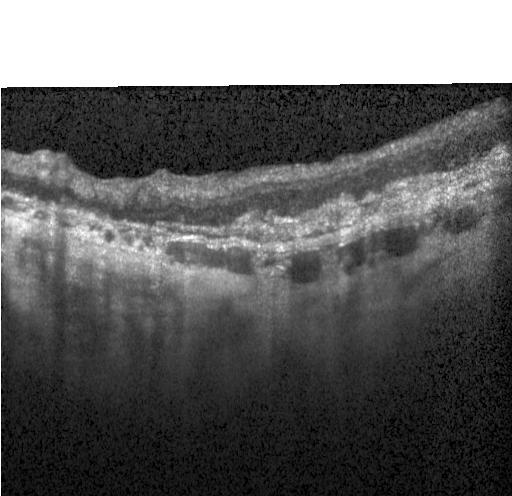

Spectral-domain optical coherence tomography. Fovea-centered. Retinal OCT cross-section.
Diagnosis: choroidal neovascularization (CNV).